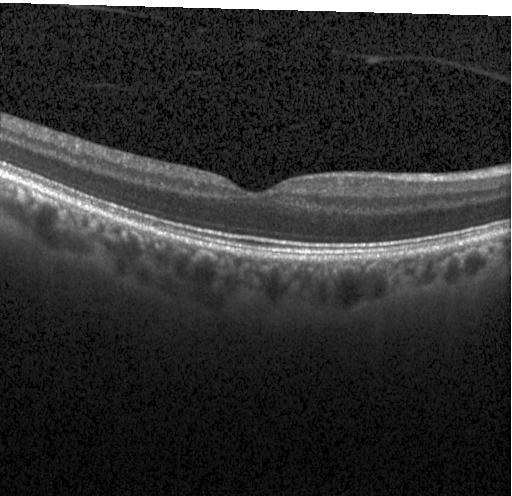

Instrument: Heidelberg Spectralis · macular scan · OCT B-scan · spectral-domain OCT.
This B-scan demonstrates no CNV, no DME, and no drusen.